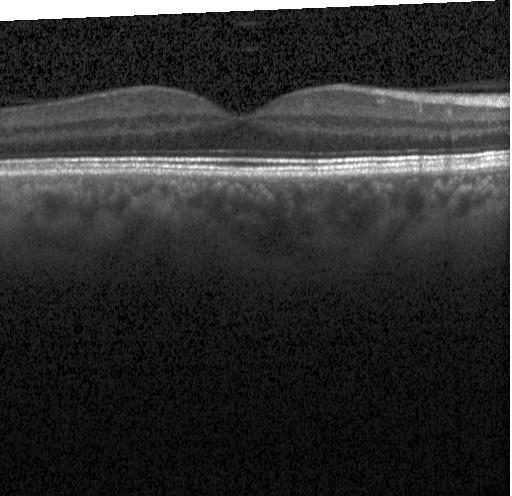 OCT finding: neither CNV, DME, nor drusen.